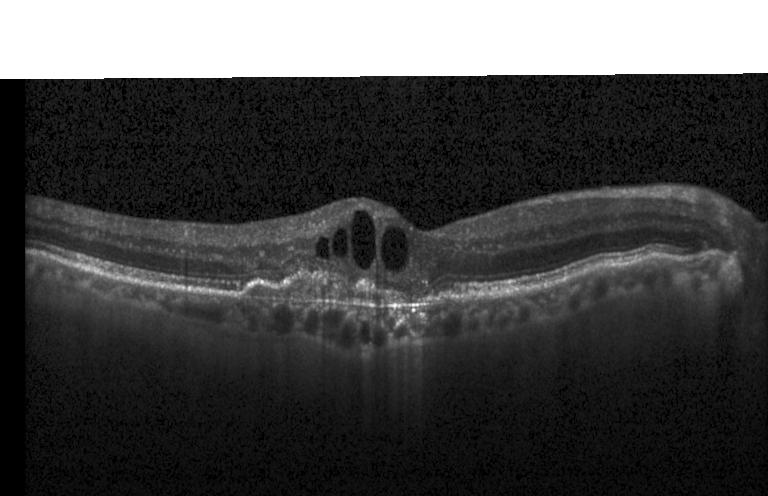 OCT B-scan showing CNV.